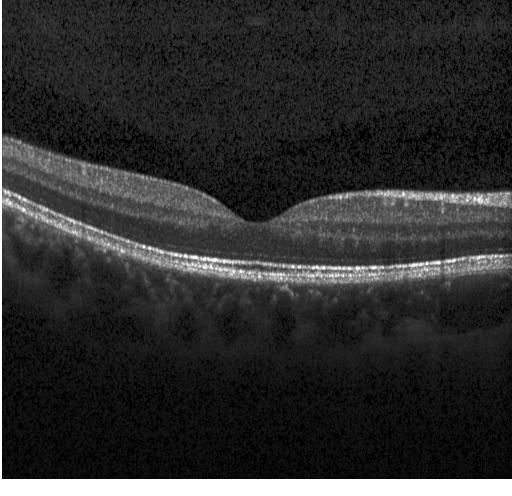 OCT finding: neither choroidal neovascularization, diabetic macular edema, nor drusen.